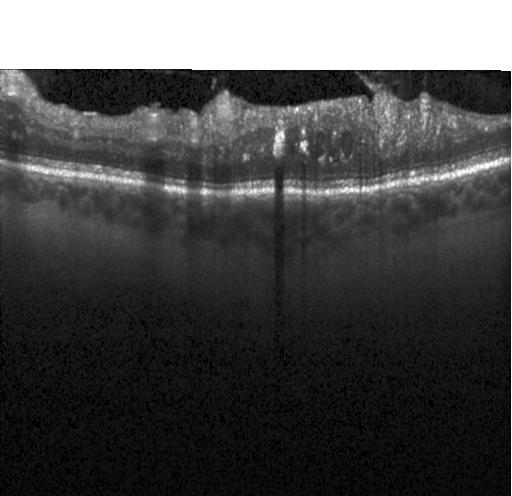
Spectral-domain OCT · optical coherence tomography scan · horizontal scan through the fovea
Diagnosis: DME.